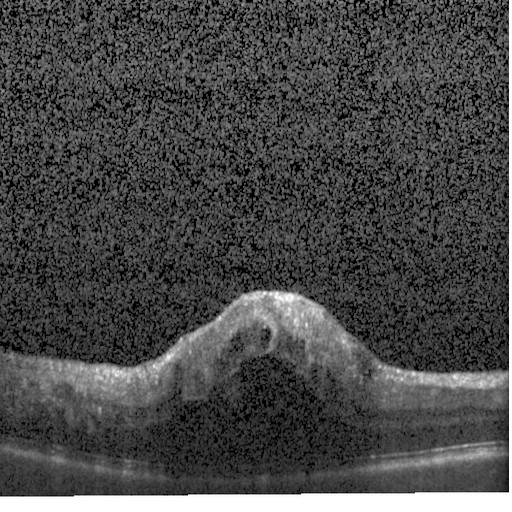 Through the macula. OCT B-scan. Acquired on a Heidelberg Spectralis.
Impression: diabetic macular edema.